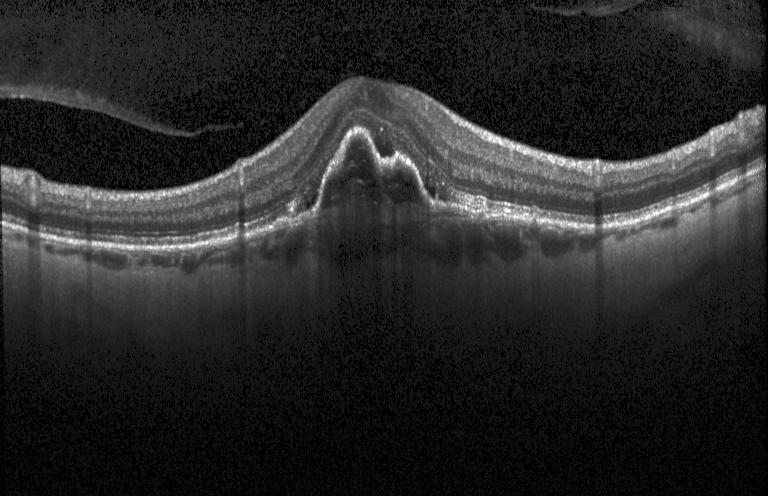
Optical coherence tomography scan, spectral-domain OCT, fovea-centered — CNV.